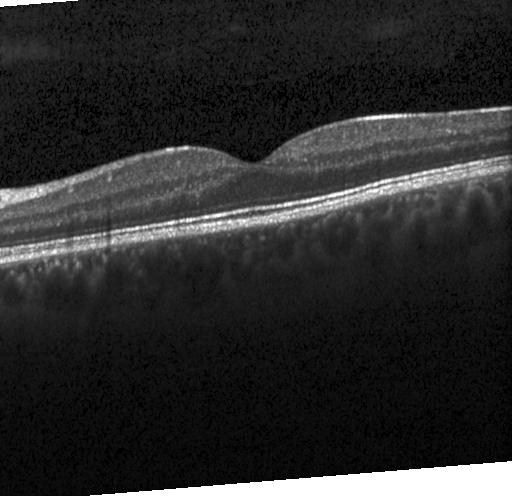
Impression: no evidence of choroidal neovascularization, diabetic macular edema, or drusen.